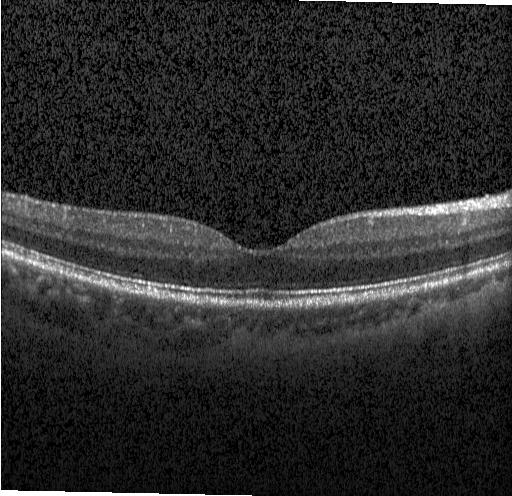

No CNV, DME, or drusen.